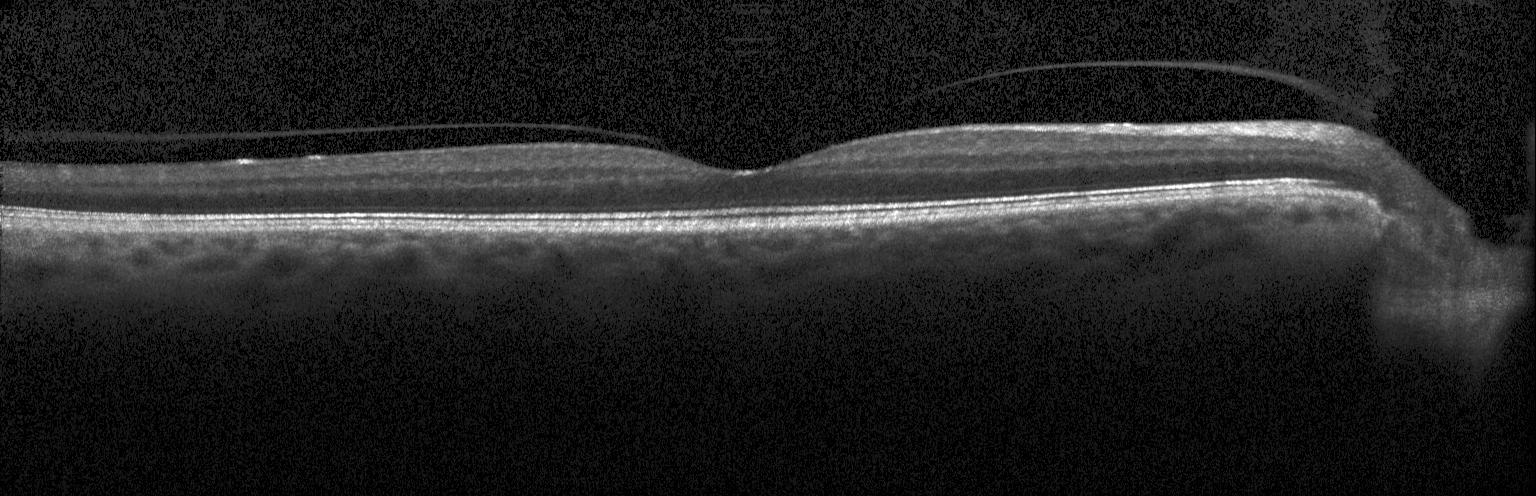

No choroidal neovascularization, no diabetic macular edema, and no drusen.